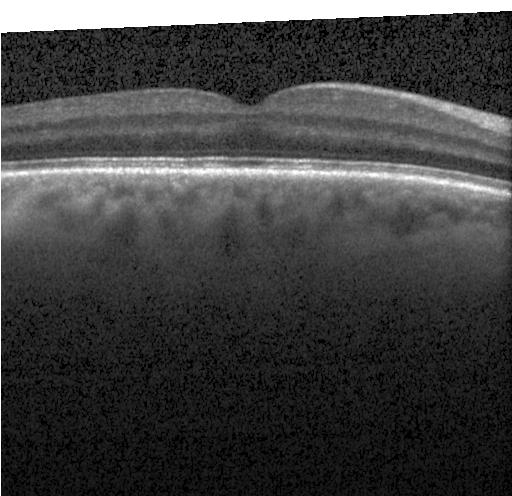

Optical coherence tomography B-scan, Heidelberg Spectralis, fovea-centered, spectral-domain optical coherence tomography — This B-scan demonstrates neither choroidal neovascularization, diabetic macular edema, nor drusen.